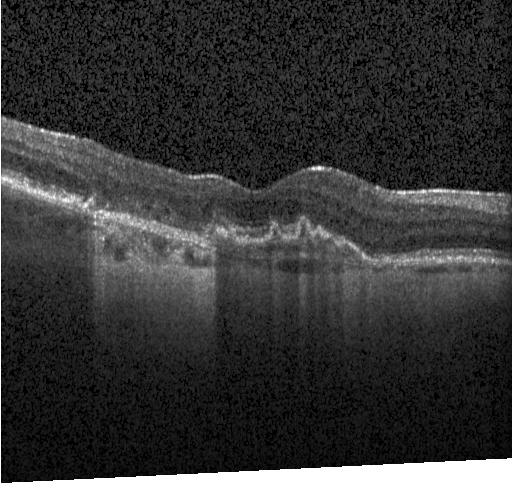

Assessment: choroidal neovascularization (CNV).